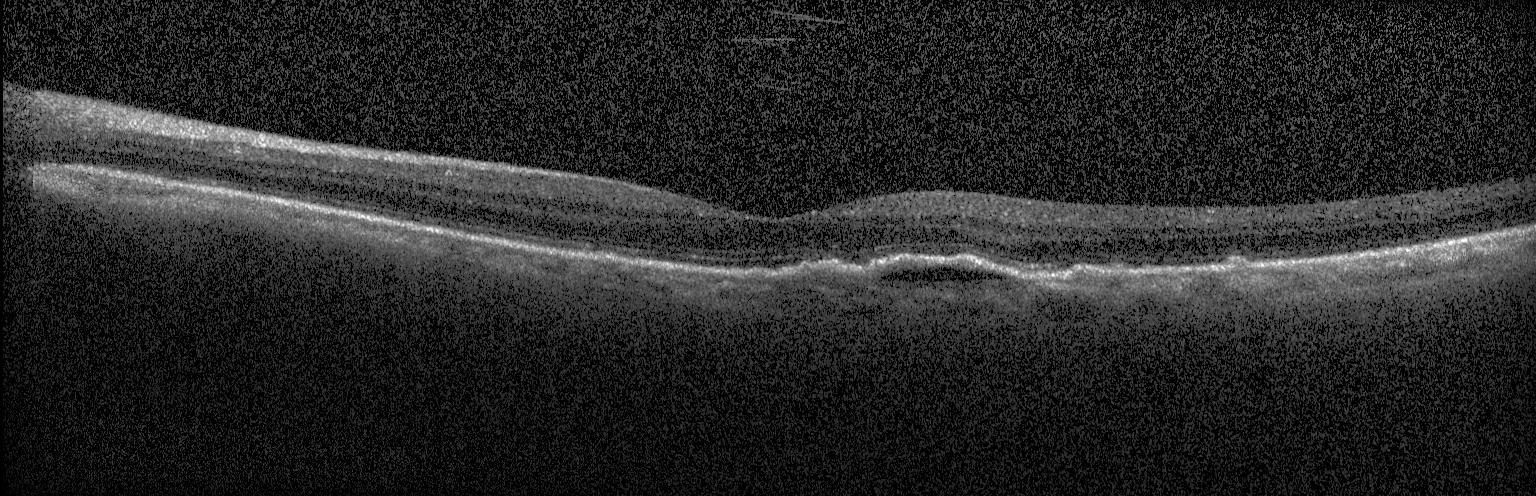
OCT scan showing CNV.